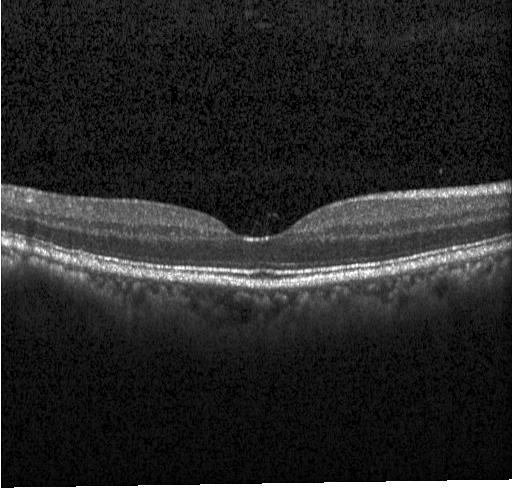 Spectral-domain OCT B-scan: no CNV, DME, or drusen.